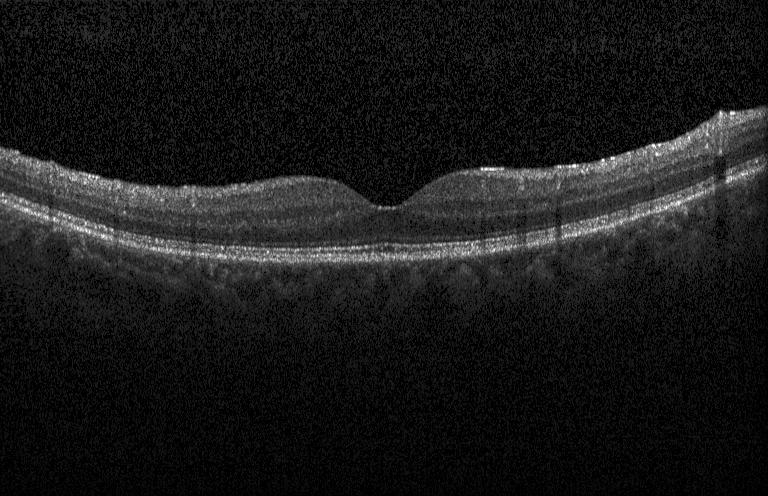 Retinal OCT cross-section — Finding: neither choroidal neovascularization, diabetic macular edema, nor drusen.